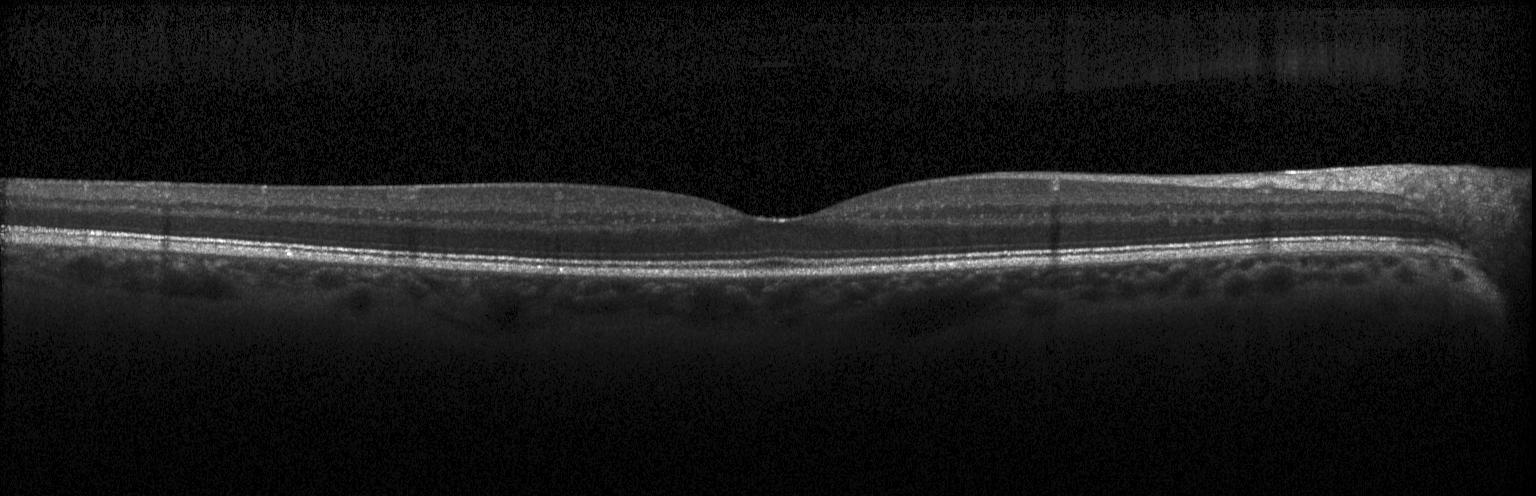

Spectral-domain OCT. Horizontal scan through the fovea. OCT line scan — Diagnosis: no evidence of choroidal neovascularization, diabetic macular edema, or drusen.